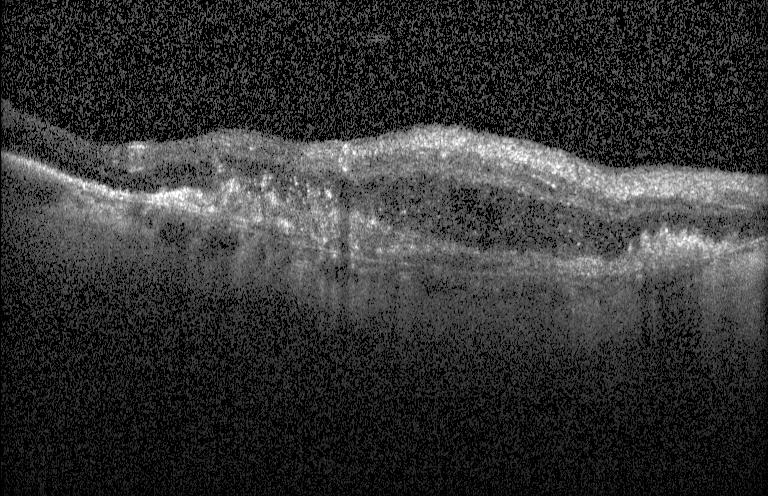 Through the macula, OCT line scan, acquired on a Heidelberg Spectralis — Macular OCT: a choroidal neovascular membrane.